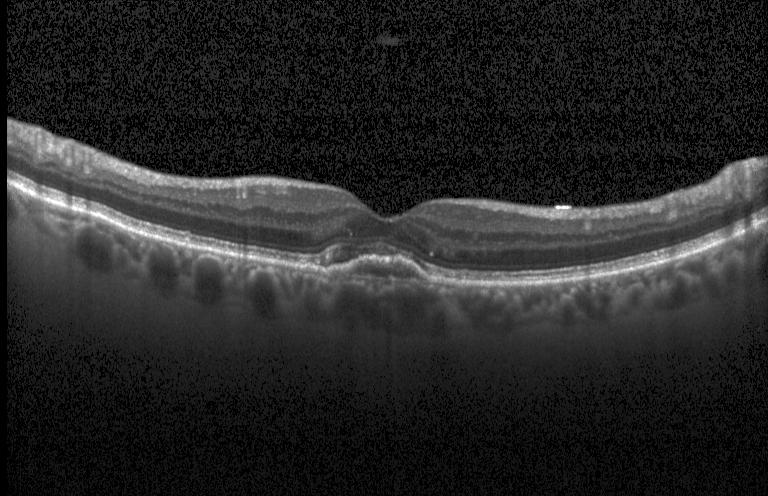

CNV.